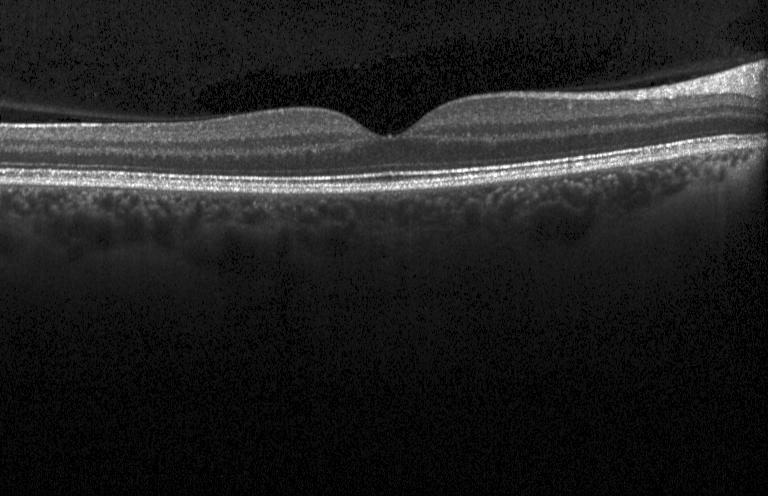

OCT finding: neither choroidal neovascularization, diabetic macular edema, nor drusen.